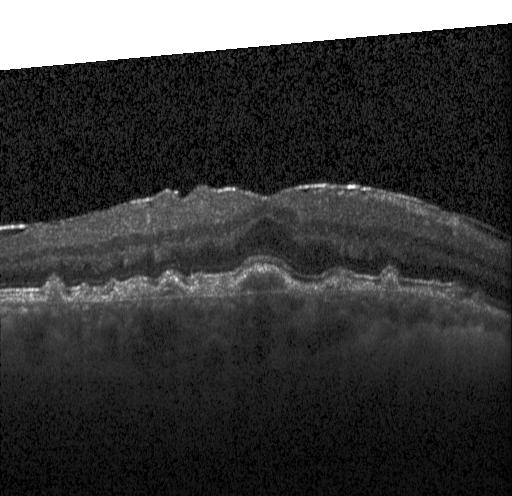
Diagnosis: CNV.